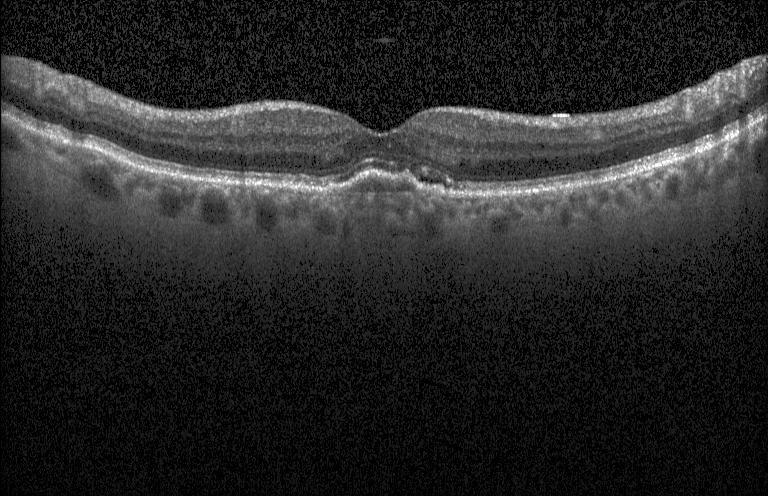
Finding: choroidal neovascularization (CNV).